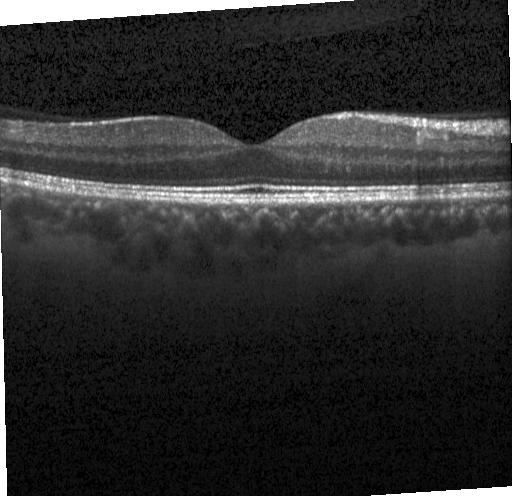

Macular OCT: no CNV, DME, or drusen.